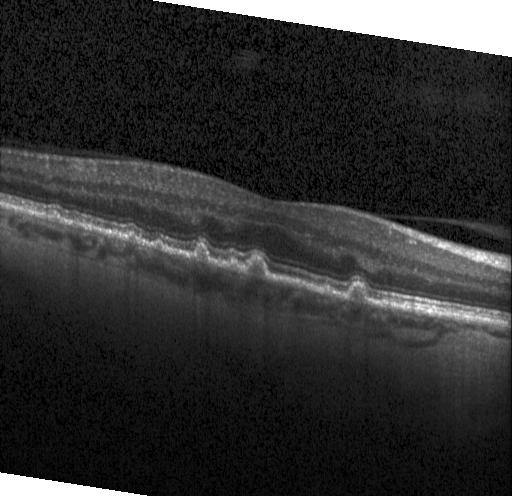

Sub-RPE drusenoid deposits.